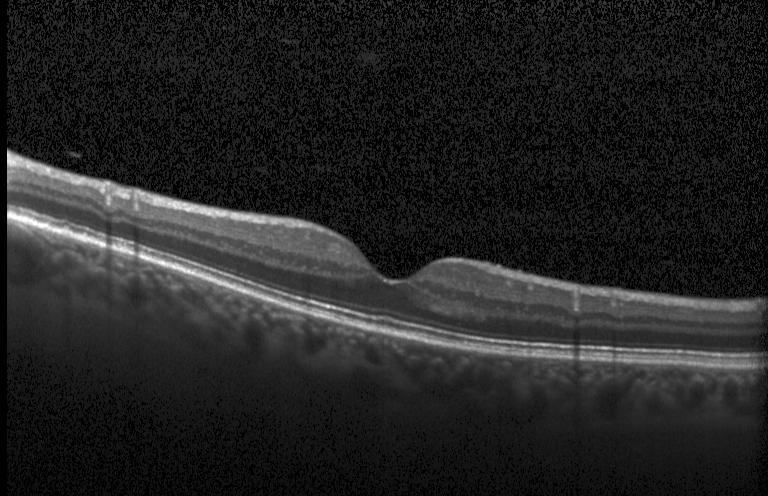
Retinal OCT B-scan; centered on the fovea; spectral-domain OCT; instrument: Heidelberg Spectralis — This B-scan demonstrates no choroidal neovascularization, diabetic macular edema, or drusen.